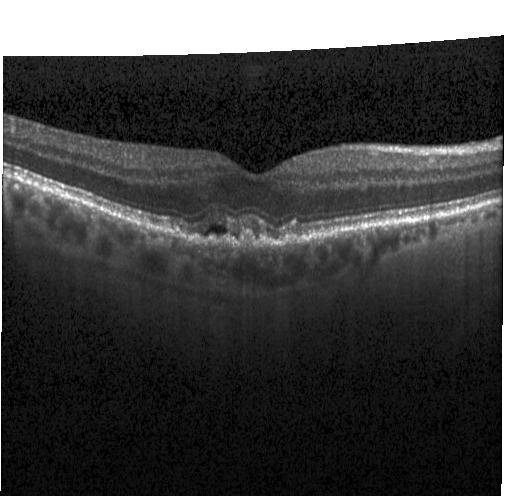

Through the macula, Heidelberg Spectralis, optical coherence tomography scan, SD-OCT — Finding: CNV.